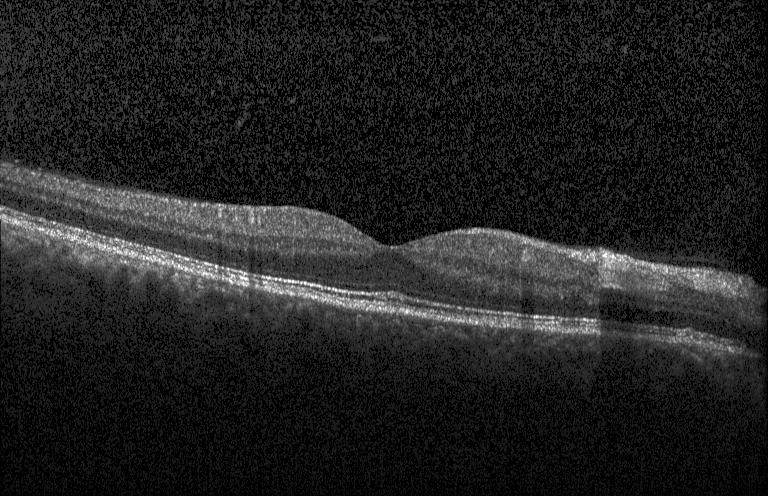
Impression: no choroidal neovascularization, diabetic macular edema, or drusen.